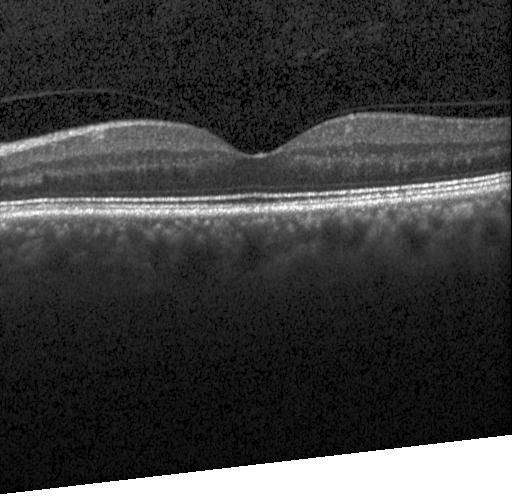
Finding: no CNV, DME, or drusen.